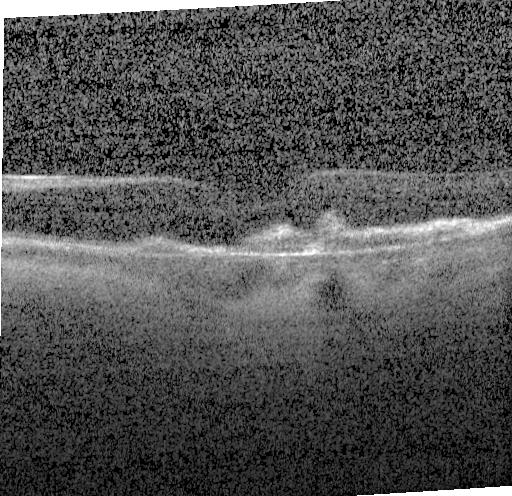
Spectral-domain OCT B-scan: a choroidal neovascular membrane.